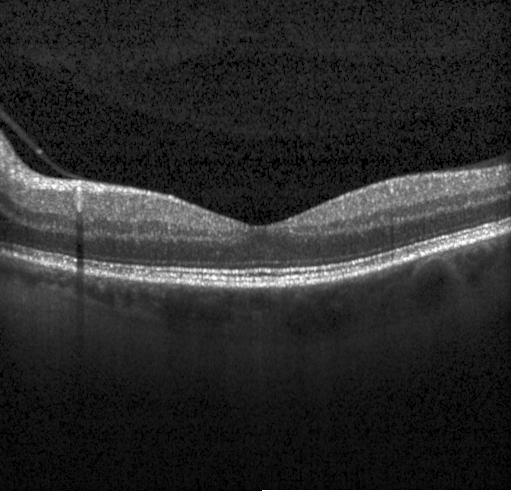

SD-OCT. OCT line scan. Heidelberg Spectralis OCT system. Dx: no CNV, DME, or drusen.